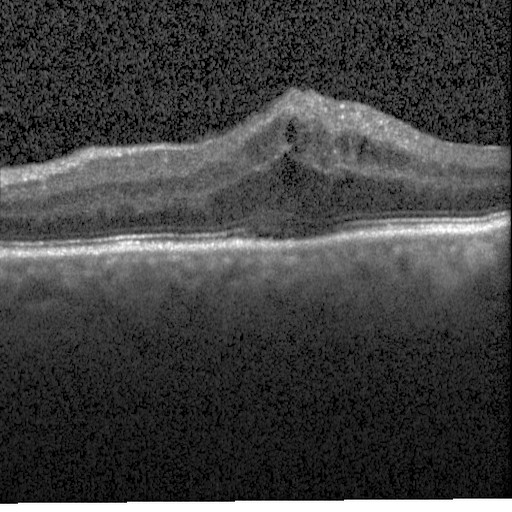 OCT finding: diabetic macular edema (DME).